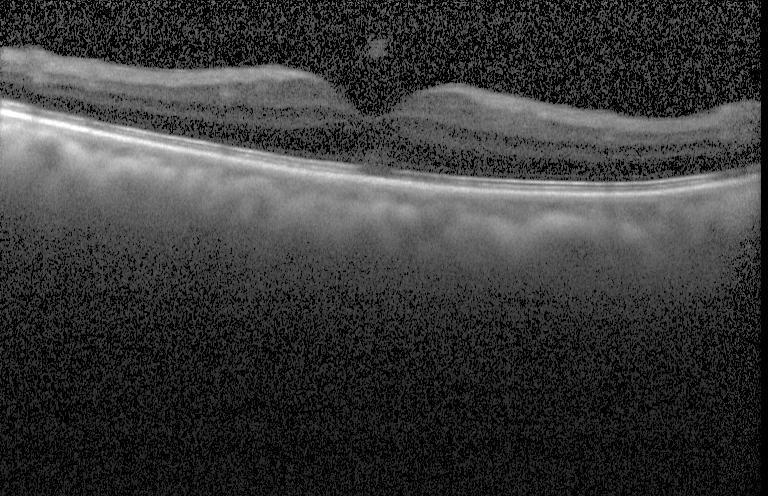

SD-OCT. Heidelberg Spectralis OCT system. Horizontal scan through the fovea. OCT line scan
Dx: choroidal neovascularization.